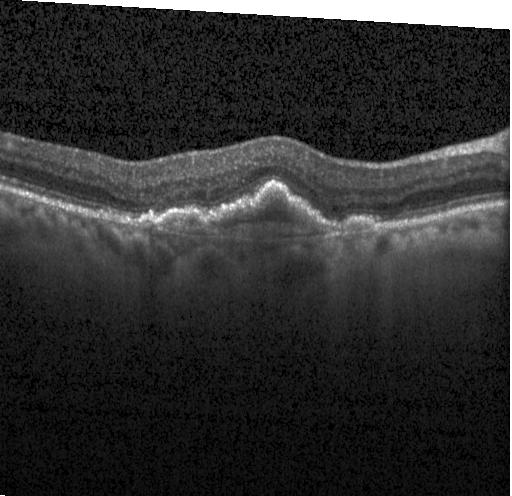

Finding: CNV.